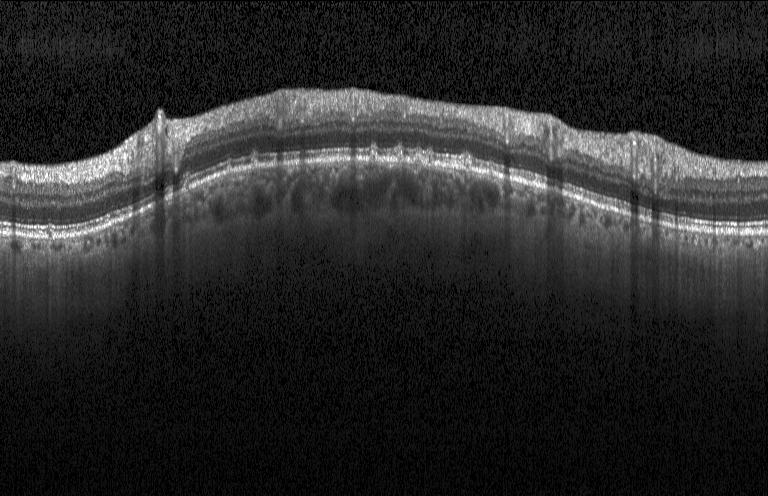 Through the macula, OCT line scan
OCT finding: multiple drusen.